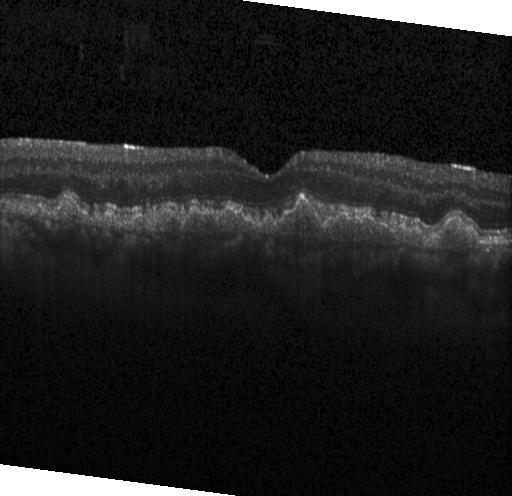

Optical coherence tomography scan · spectral-domain OCT · Heidelberg Spectralis OCT system.
Finding: choroidal neovascularization.